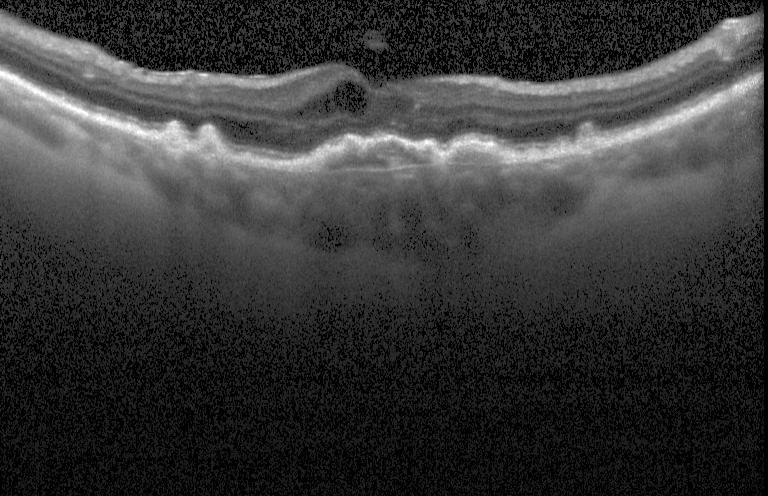
OCT B-scan; fovea-centered. Impression: a choroidal neovascular membrane.